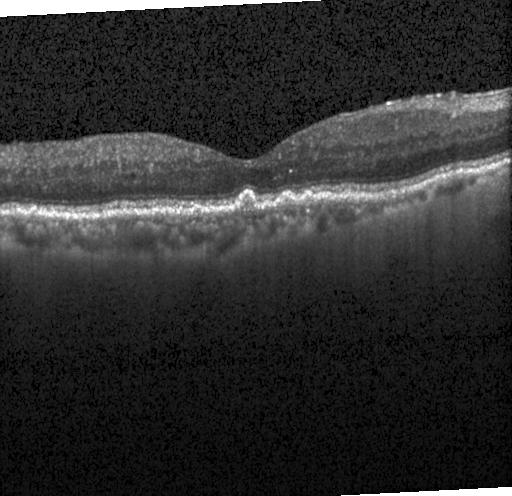
OCT line scan. Horizontal scan through the fovea.
Impression: multiple drusen.